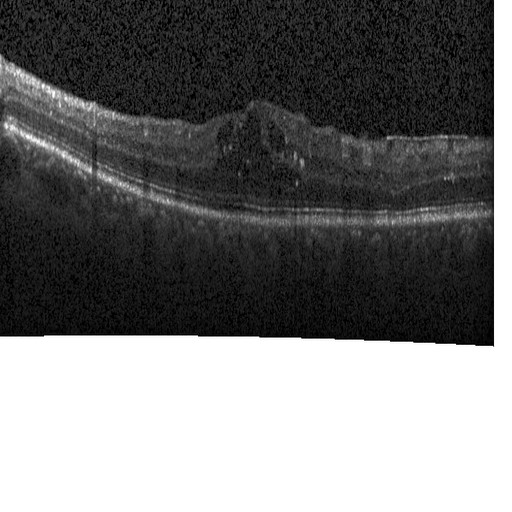 Centered on the fovea. Heidelberg Spectralis OCT system. Retinal OCT cross-section. Spectral-domain optical coherence tomography
Diabetic macular edema (DME).